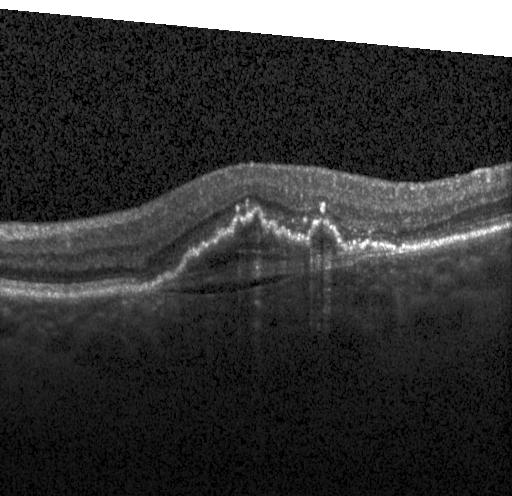

Retinal OCT B-scan.
Assessment: a choroidal neovascular membrane.